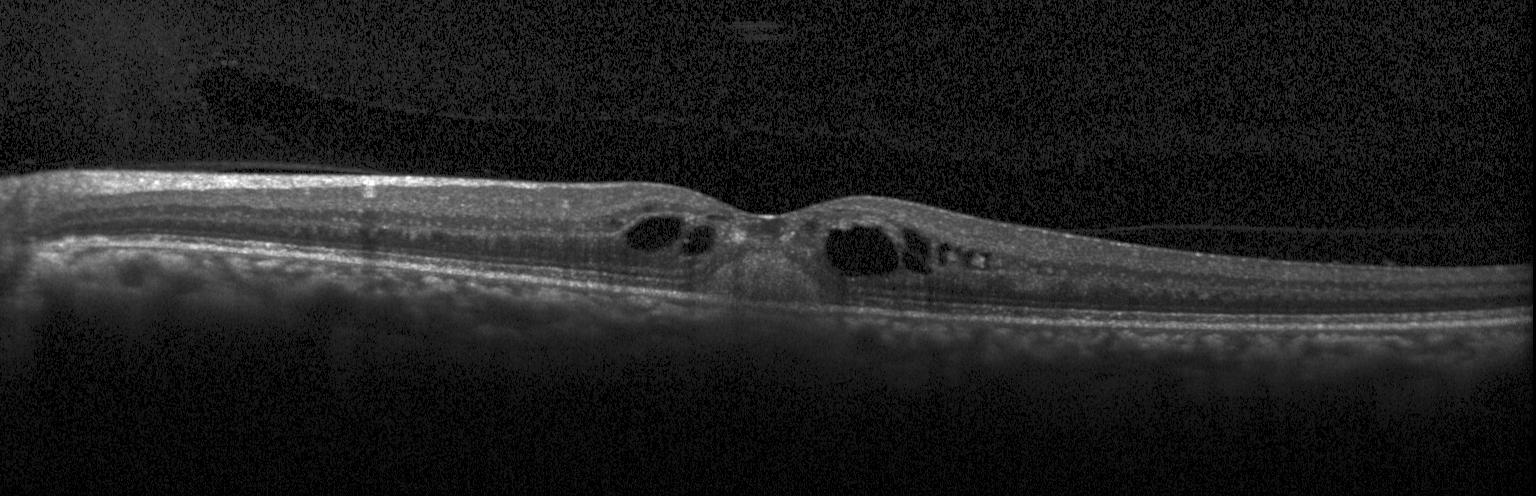 Retinal OCT B-scan. This B-scan demonstrates a choroidal neovascular membrane.